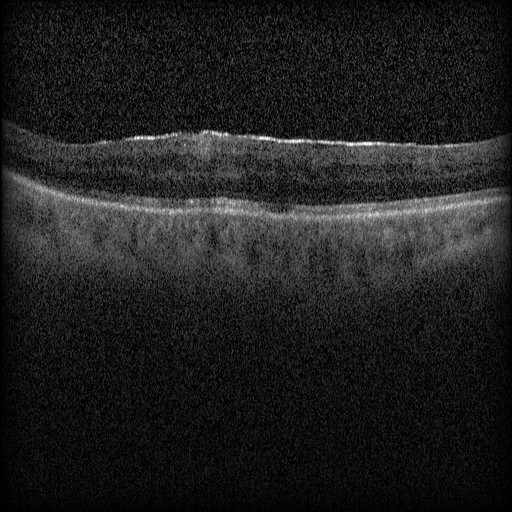 OCT line scan
Impression: diabetic macular edema (DME).